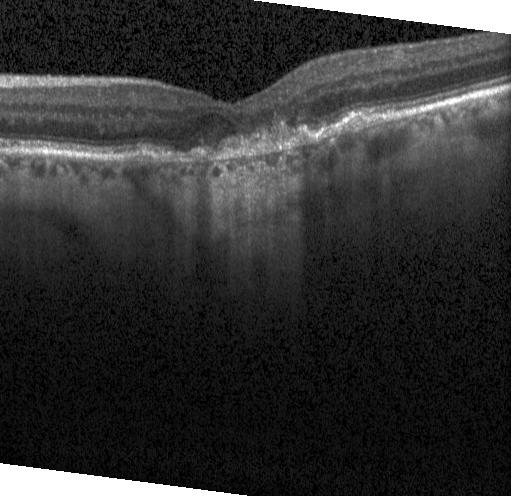
Macular OCT: a choroidal neovascular membrane.